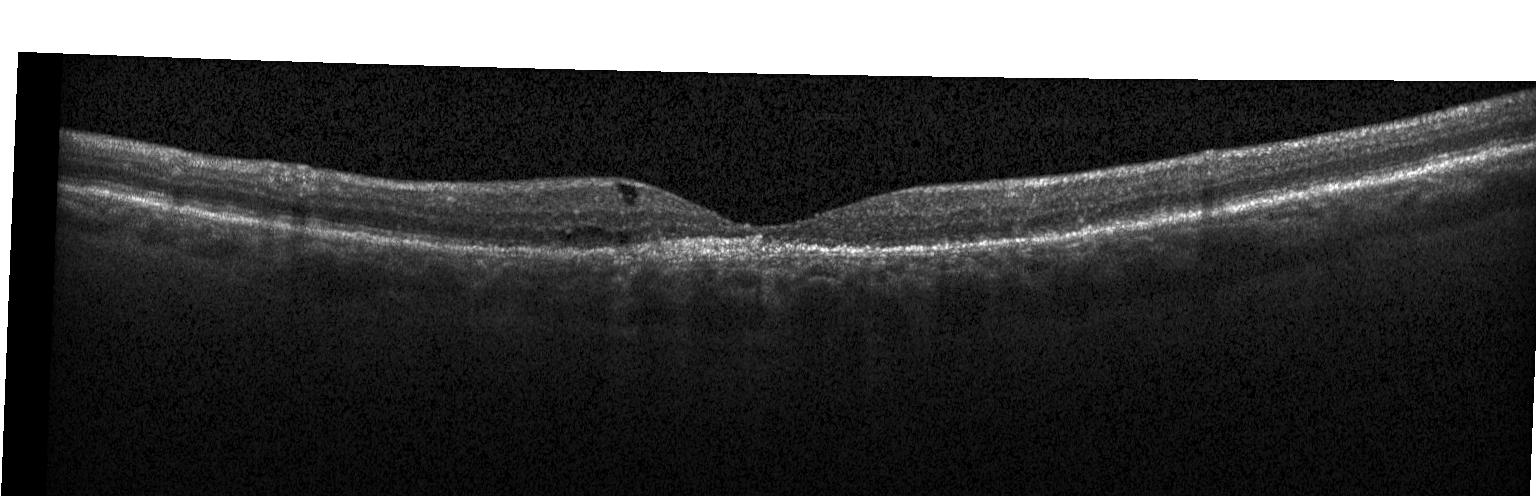
Acquired on a Heidelberg Spectralis; OCT line scan; spectral-domain optical coherence tomography; through the macula — OCT finding: CNV.